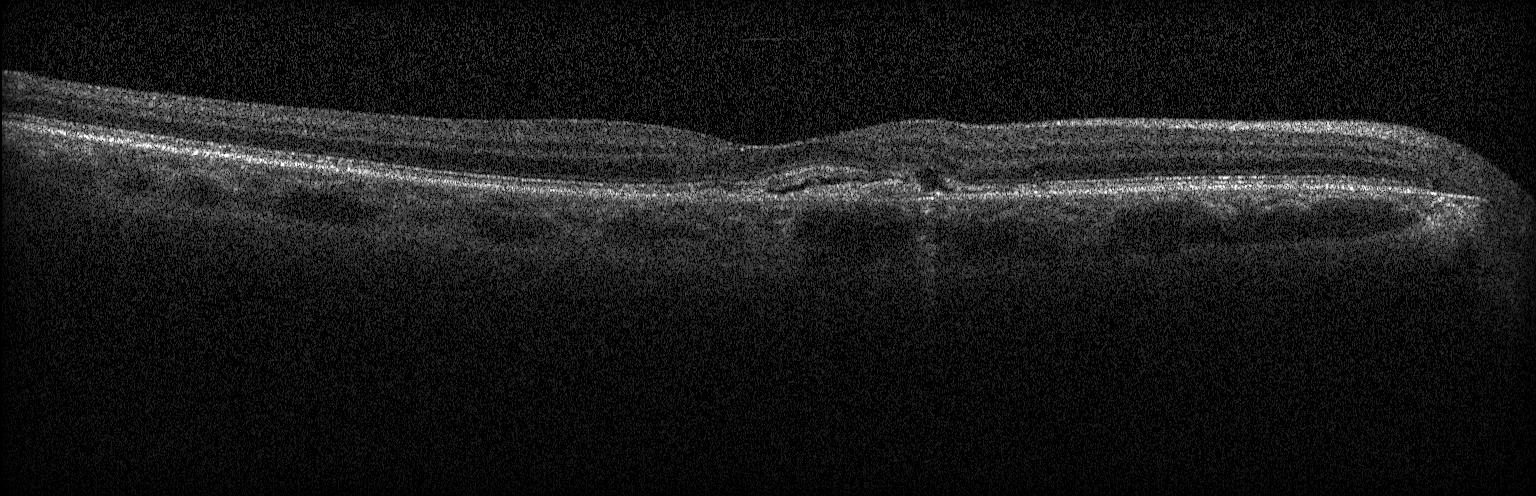 SD-OCT · optical coherence tomography scan. Finding: choroidal neovascularization.